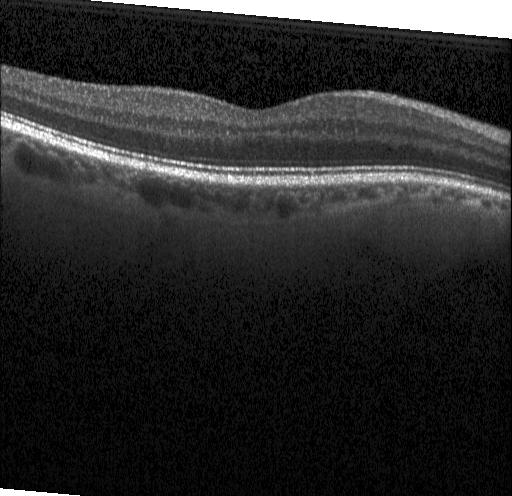 Heidelberg Spectralis OCT system. Spectral-domain OCT. Through the macula. OCT line scan. Impression: no evidence of choroidal neovascularization, diabetic macular edema, or drusen.